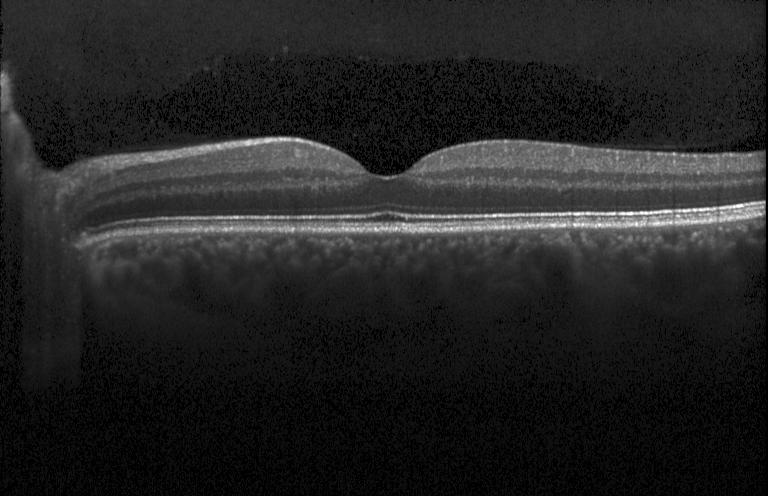

No CNV, no DME, and no drusen.